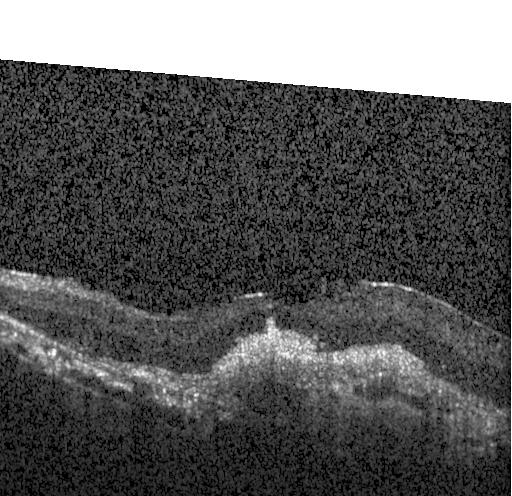

Choroidal neovascularization.